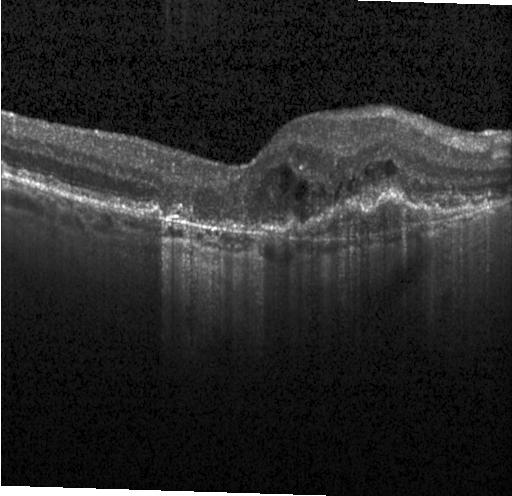
Heidelberg Spectralis OCT system, spectral-domain OCT, retinal OCT B-scan, macular scan.
OCT finding: a choroidal neovascular membrane.